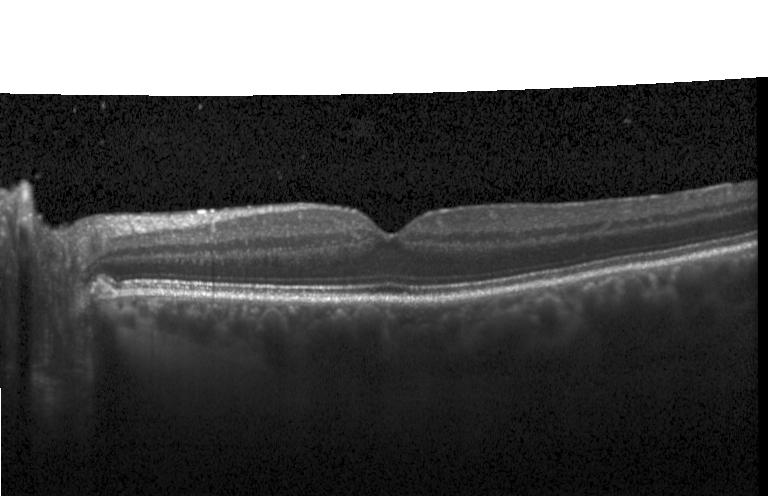
Macular OCT: no choroidal neovascularization, diabetic macular edema, or drusen.